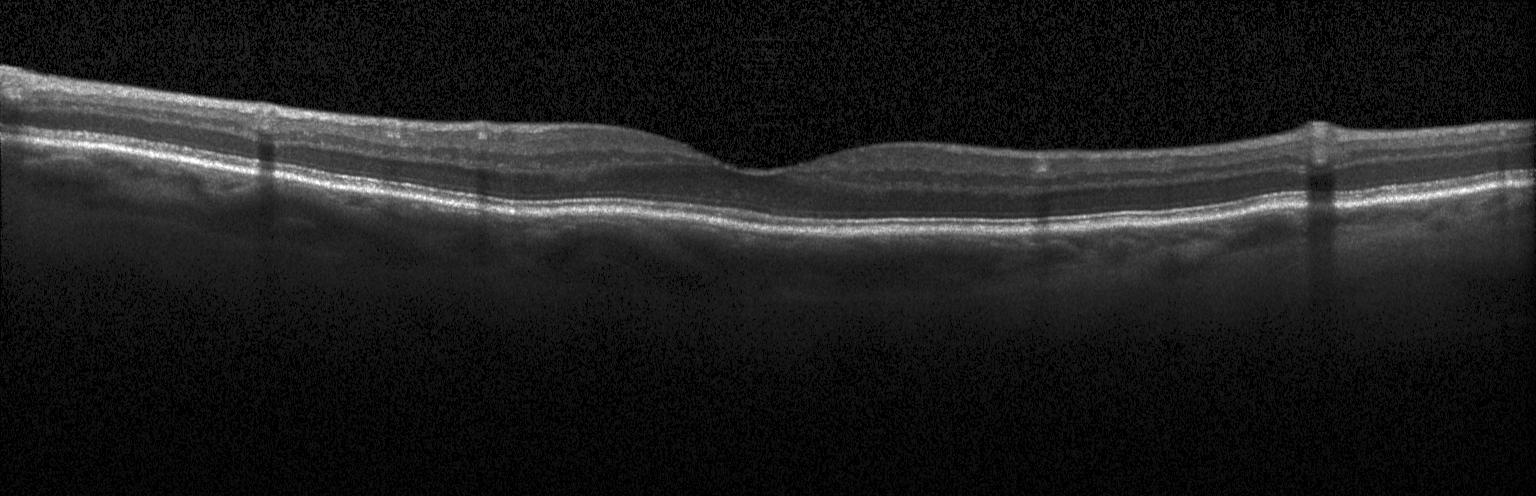 Fovea-centered, optical coherence tomography scan.
This B-scan demonstrates no evidence of choroidal neovascularization, diabetic macular edema, or drusen.